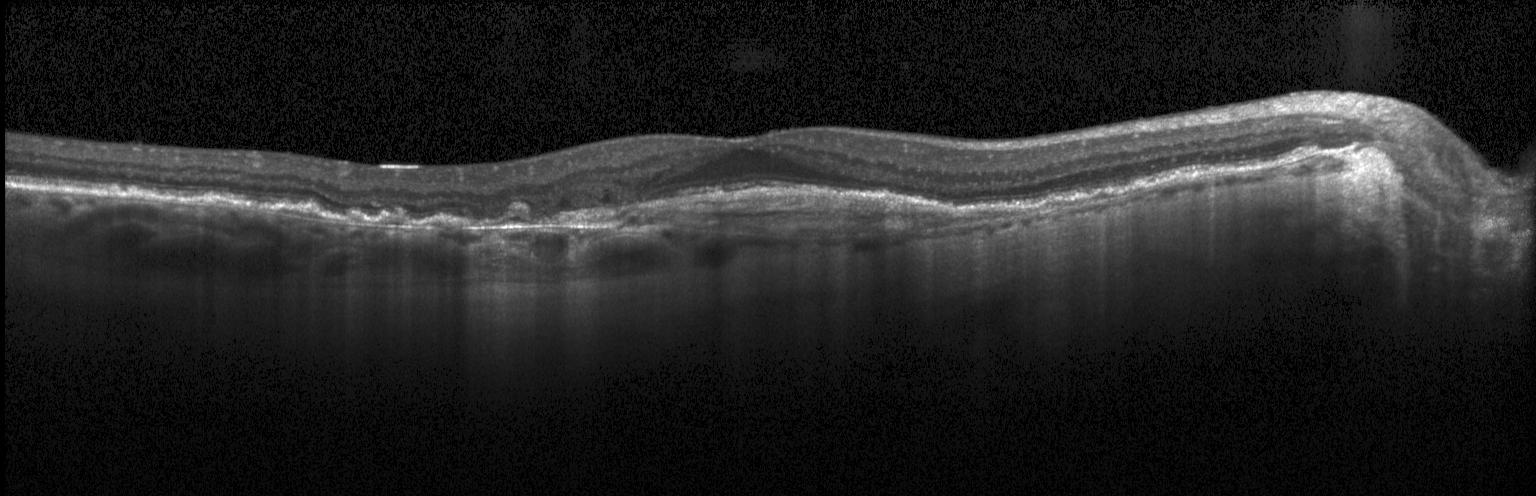
Optical coherence tomography B-scan · horizontal scan through the fovea.
A choroidal neovascular membrane.